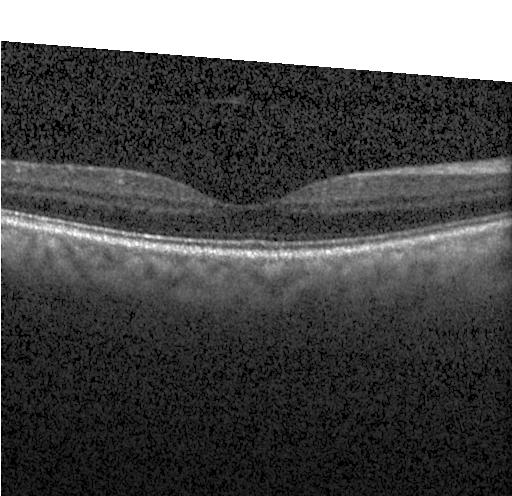

Retinal OCT cross-section, instrument: Heidelberg Spectralis, SD-OCT, fovea-centered — No evidence of CNV, DME, or drusen.